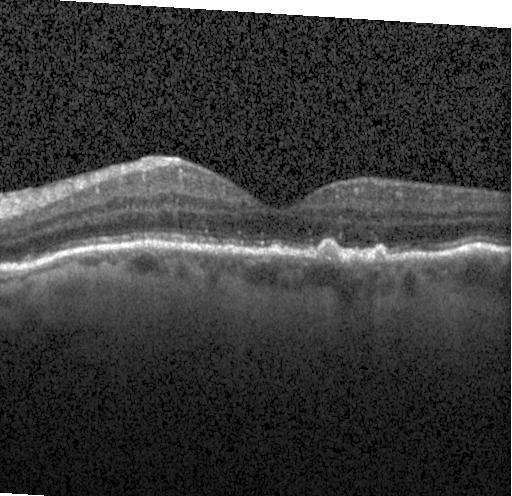

Optical coherence tomography B-scan, spectral-domain optical coherence tomography — Finding: sub-RPE drusenoid deposits.